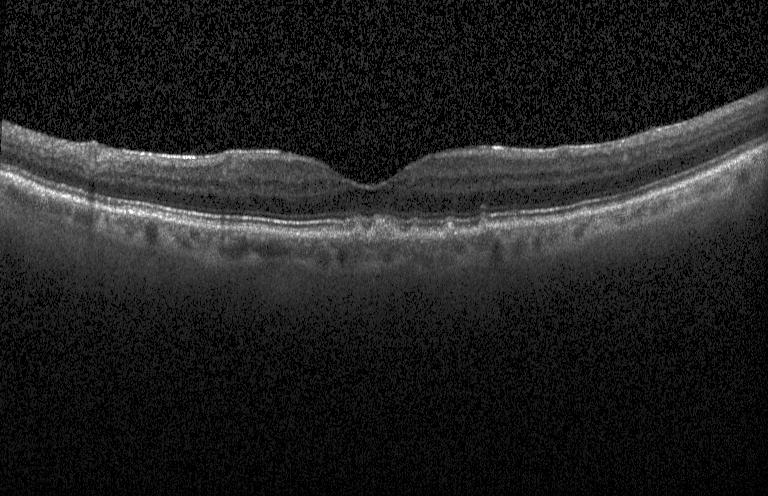

Macular OCT: sub-RPE drusenoid deposits.